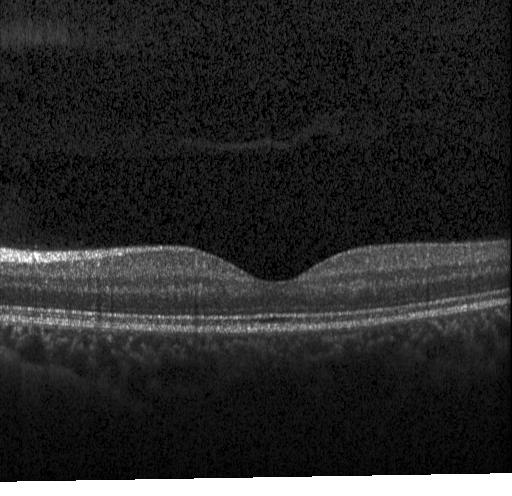 Finding: no evidence of choroidal neovascularization, diabetic macular edema, or drusen.